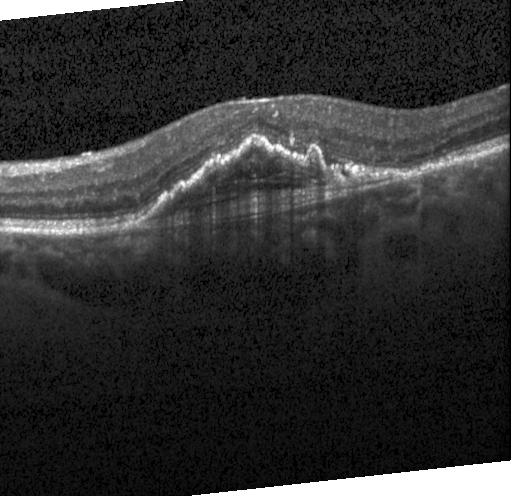
Finding: choroidal neovascularization (CNV).